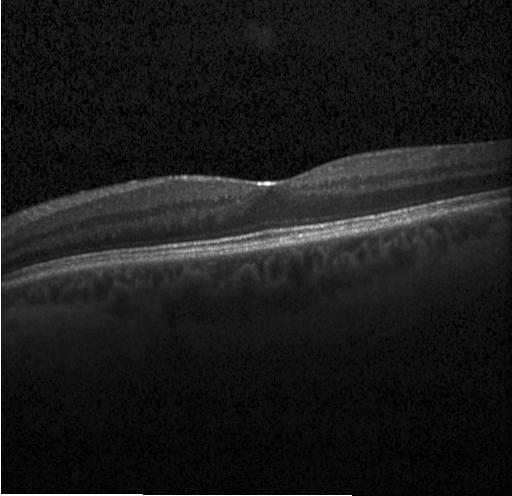 Dx: no choroidal neovascularization, diabetic macular edema, or drusen.